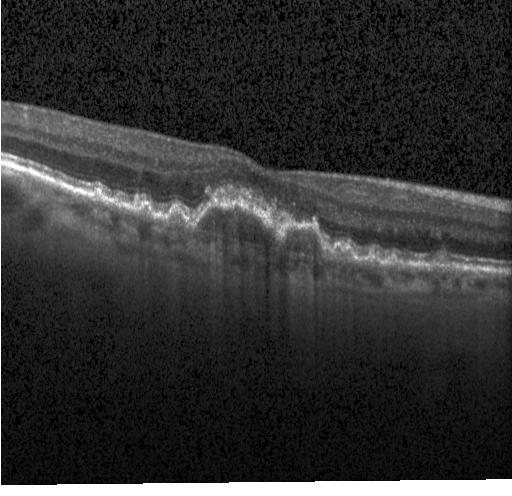

Retinal OCT cross-section
OCT finding: choroidal neovascularization (CNV).